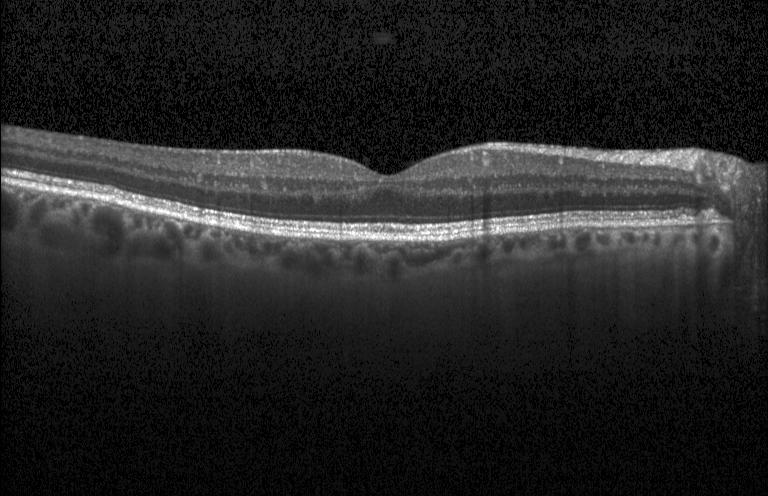

Optical coherence tomography scan · SD-OCT
Dx: no evidence of CNV, DME, or drusen.